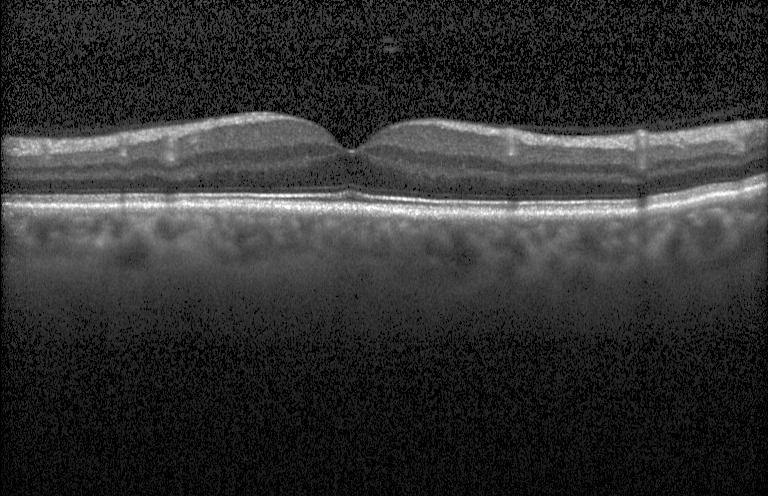 Macular scan, retinal OCT cross-section — Impression: neither choroidal neovascularization, diabetic macular edema, nor drusen.